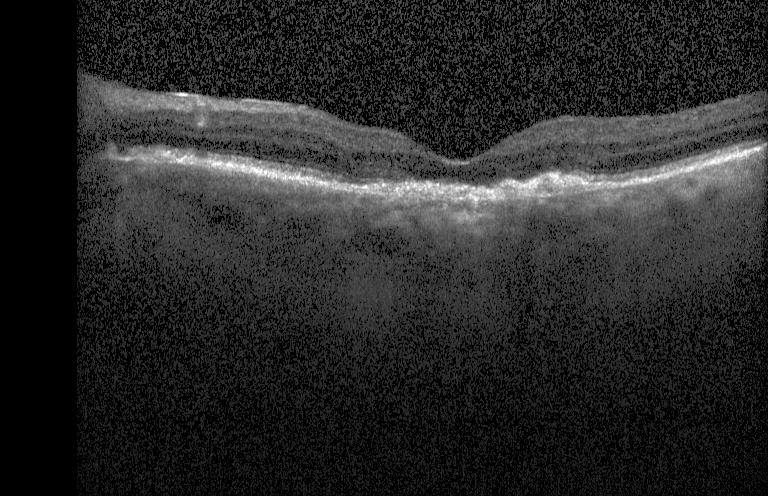 OCT finding: choroidal neovascularization.